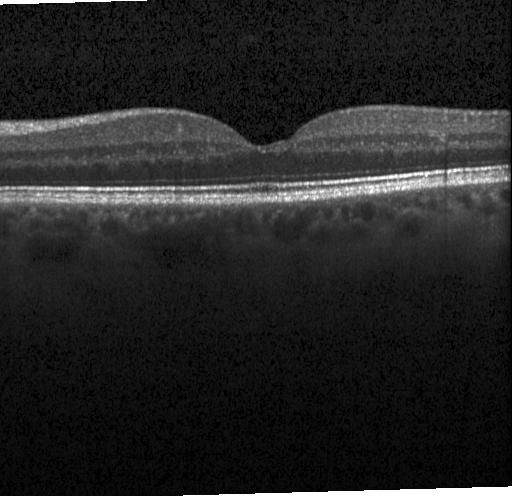 Diagnosis: no CNV, no DME, and no drusen.